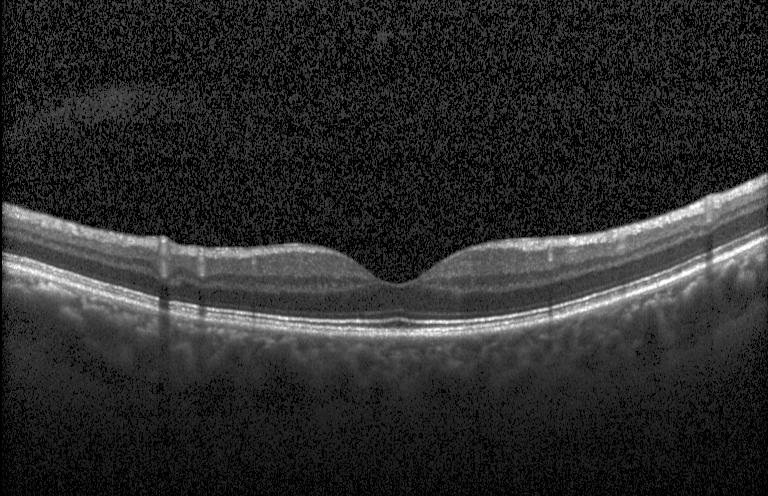
Dx: no choroidal neovascularization, diabetic macular edema, or drusen.